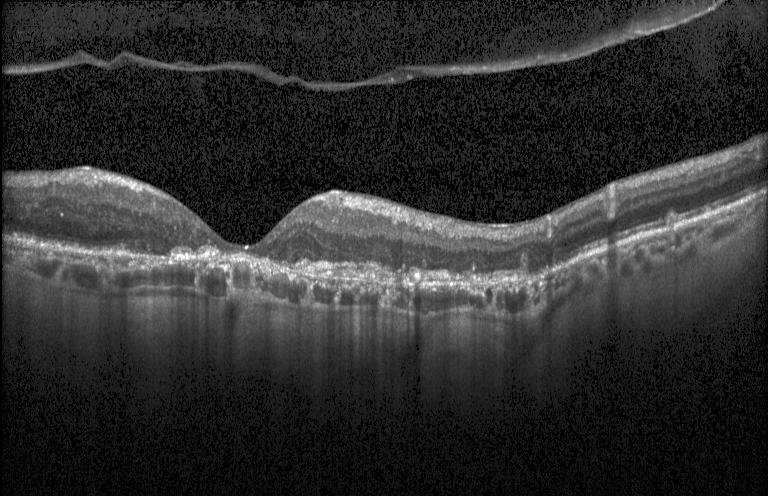

This B-scan demonstrates choroidal neovascularization.